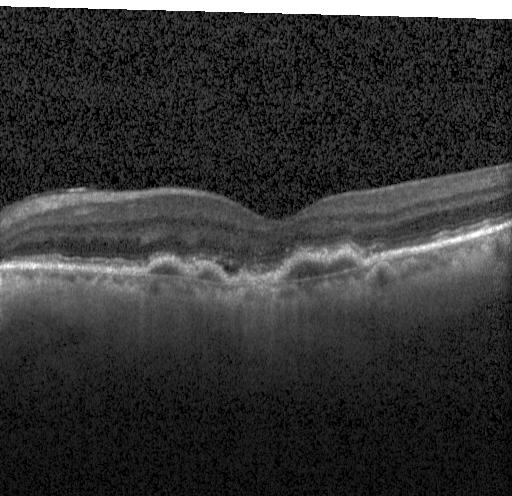
Retinal OCT cross-section, acquired on a Heidelberg Spectralis.
Dx: a choroidal neovascular membrane.